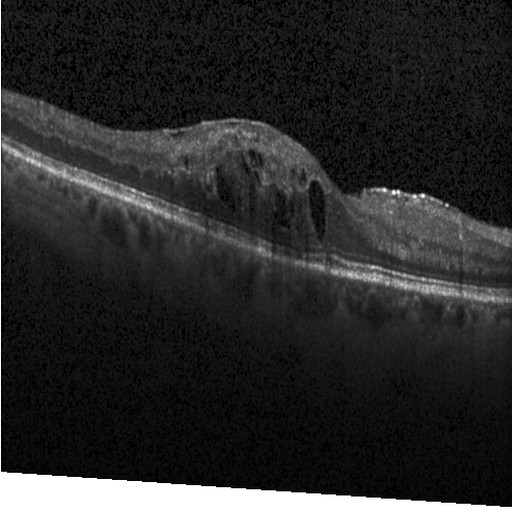 SD-OCT; OCT B-scan.
Diagnosis: DME.